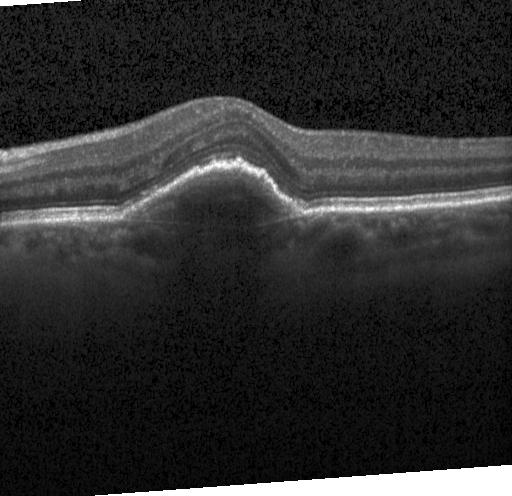
OCT line scan
Diagnosis: choroidal neovascularization.